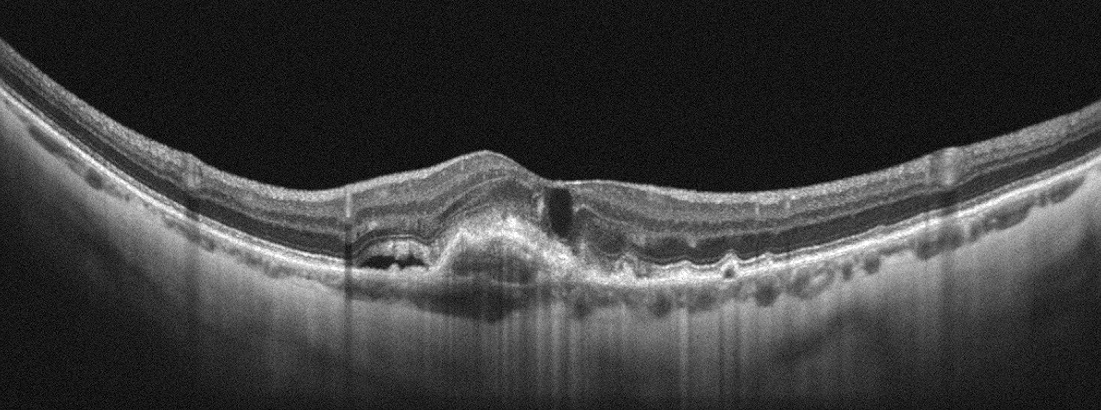
Macular OCT demonstrating age-related macular degeneration (AMD).